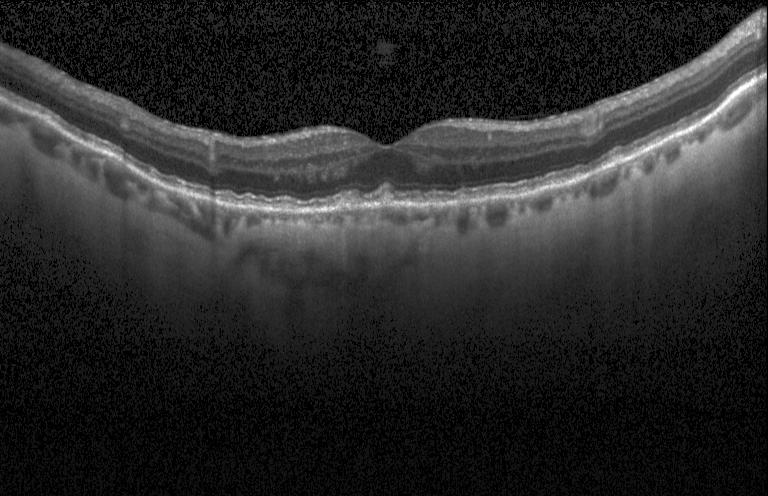

Optical coherence tomography B-scan, Heidelberg Spectralis OCT system, horizontal scan through the fovea.
OCT finding: drusen.